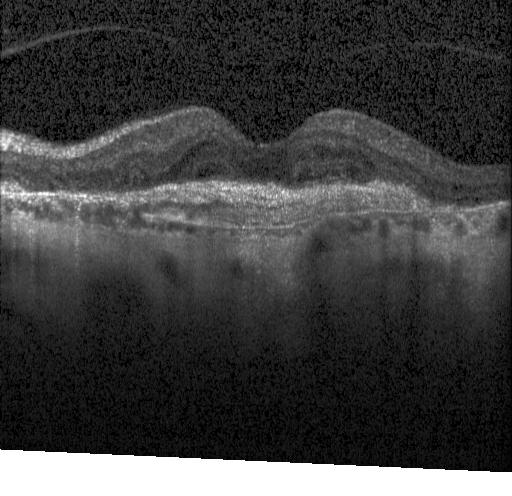
Retinal OCT B-scan. This B-scan demonstrates a choroidal neovascular membrane.